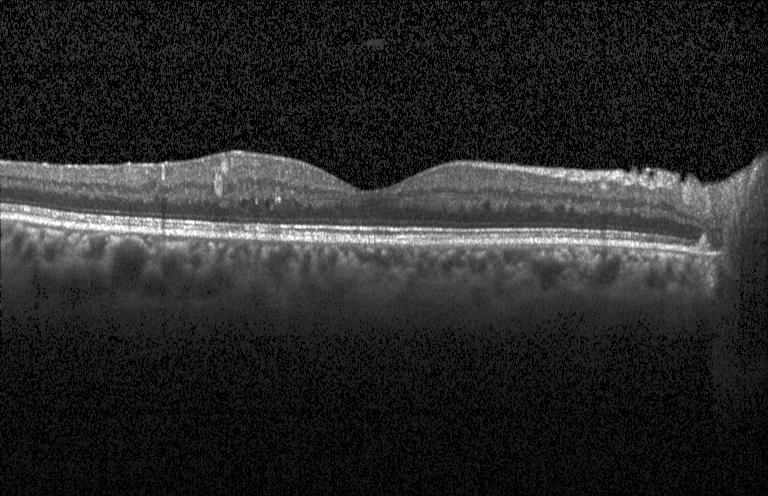

Retinal OCT cross-section showing DME.